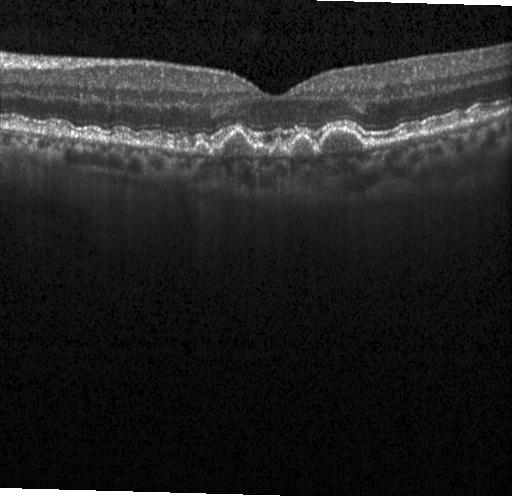
Fovea-centered, optical coherence tomography B-scan. The scan shows multiple drusen.